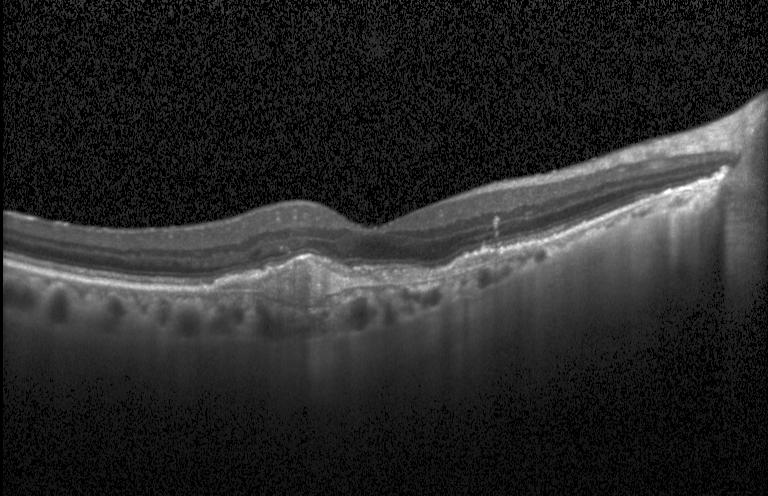
Retinal OCT B-scan. Impression: a choroidal neovascular membrane.